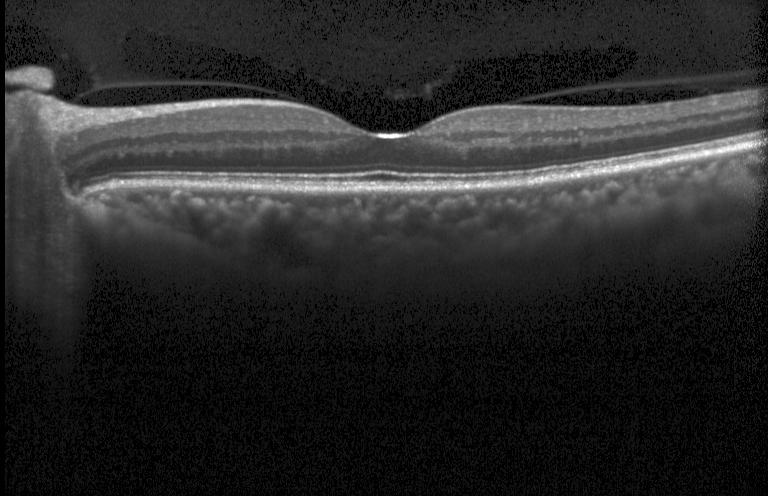

Optical coherence tomography B-scan · SD-OCT
Finding: no choroidal neovascularization, diabetic macular edema, or drusen.